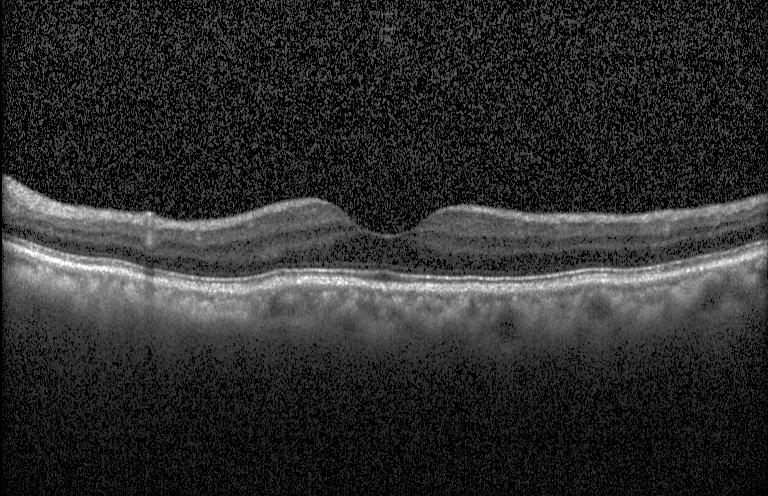
OCT line scan. Finding: no CNV, no DME, and no drusen.